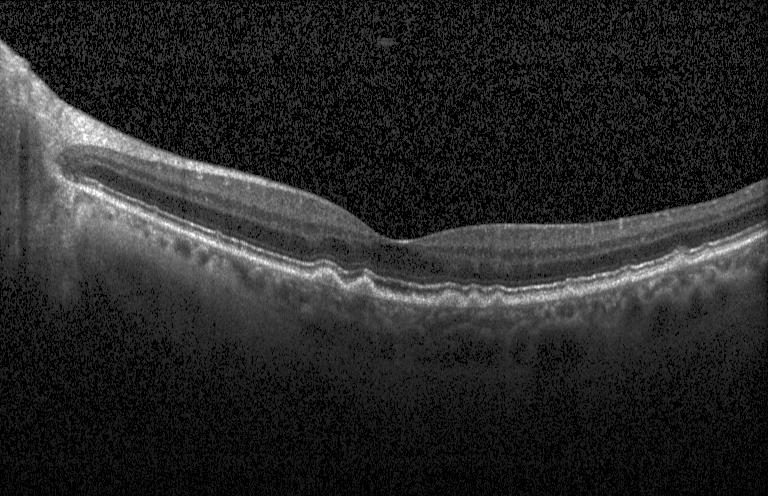

Retinal OCT B-scan. SD-OCT. Through the macula. Heidelberg Spectralis OCT system — Finding: drusen.